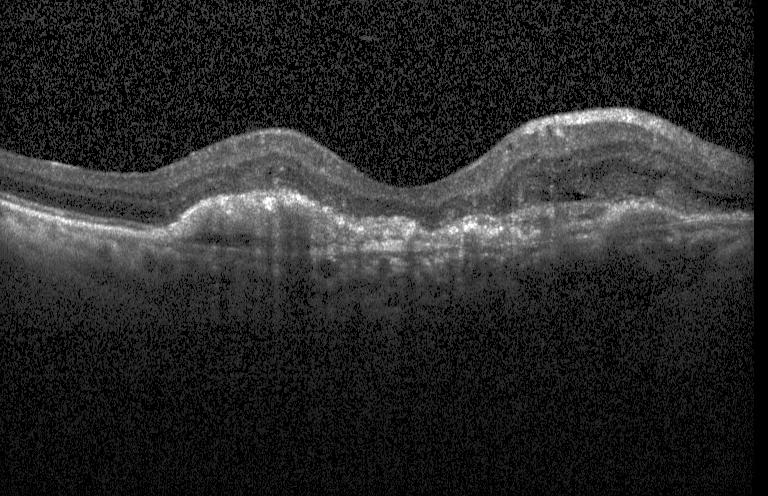
Impression: a choroidal neovascular membrane.